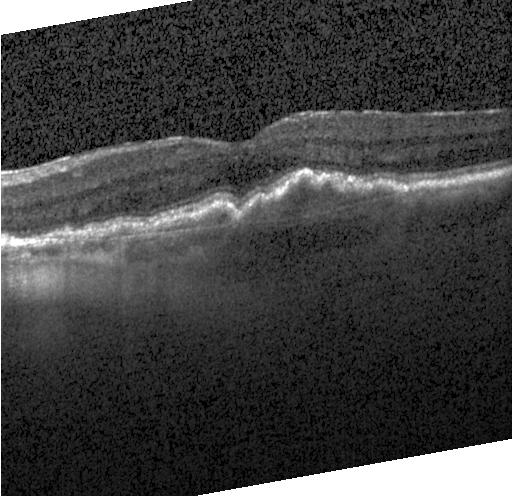 Acquired on a Heidelberg Spectralis, retinal OCT cross-section — Finding: choroidal neovascularization.